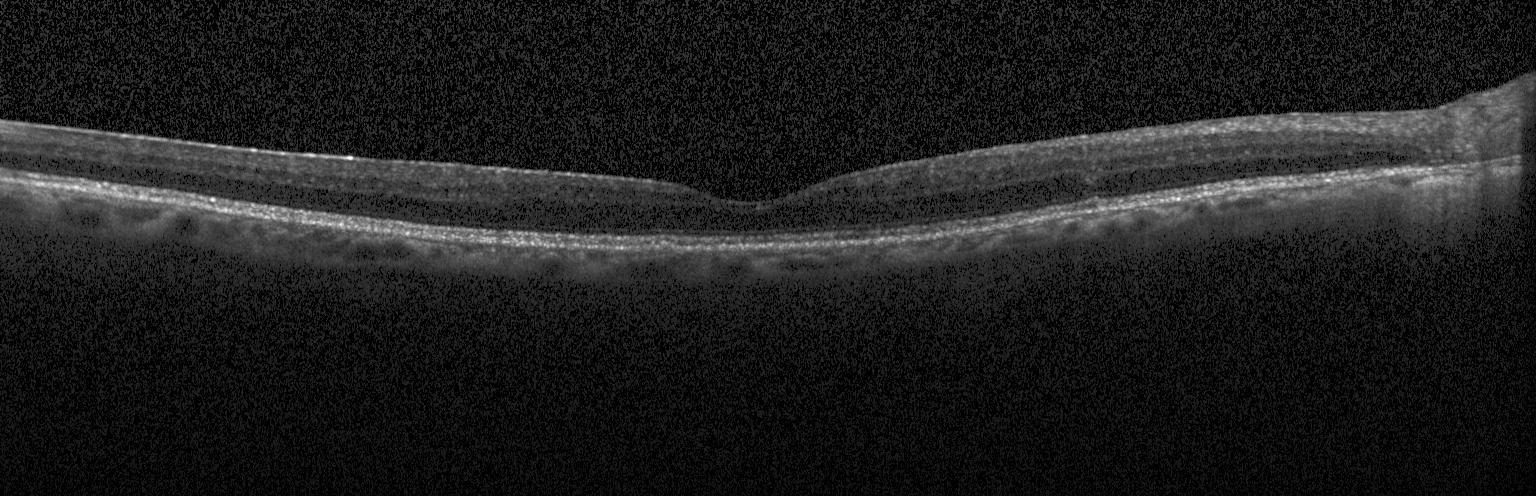

Retinal OCT cross-section; macular scan; acquired on a Heidelberg Spectralis. Impression: no CNV, DME, or drusen.